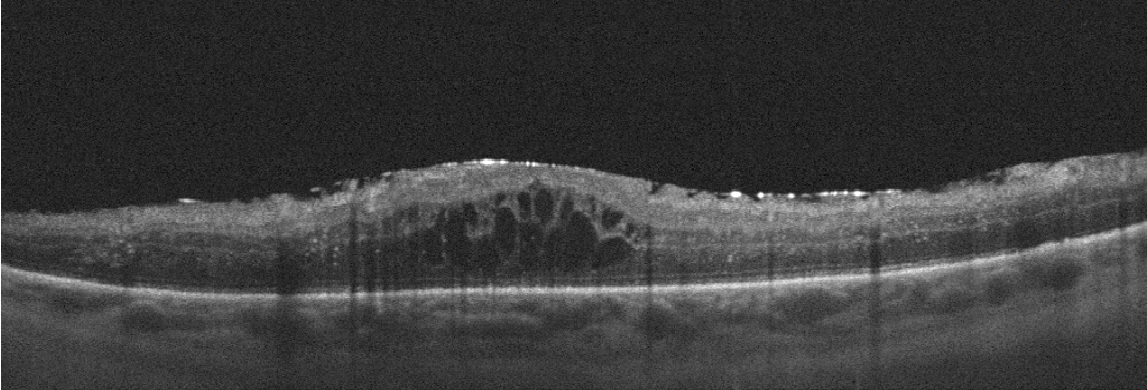

Fovea-centered; OCT line scan; acquired on an Optovue Avanti RTVue XR. Dx: diabetic macular edema (DME).